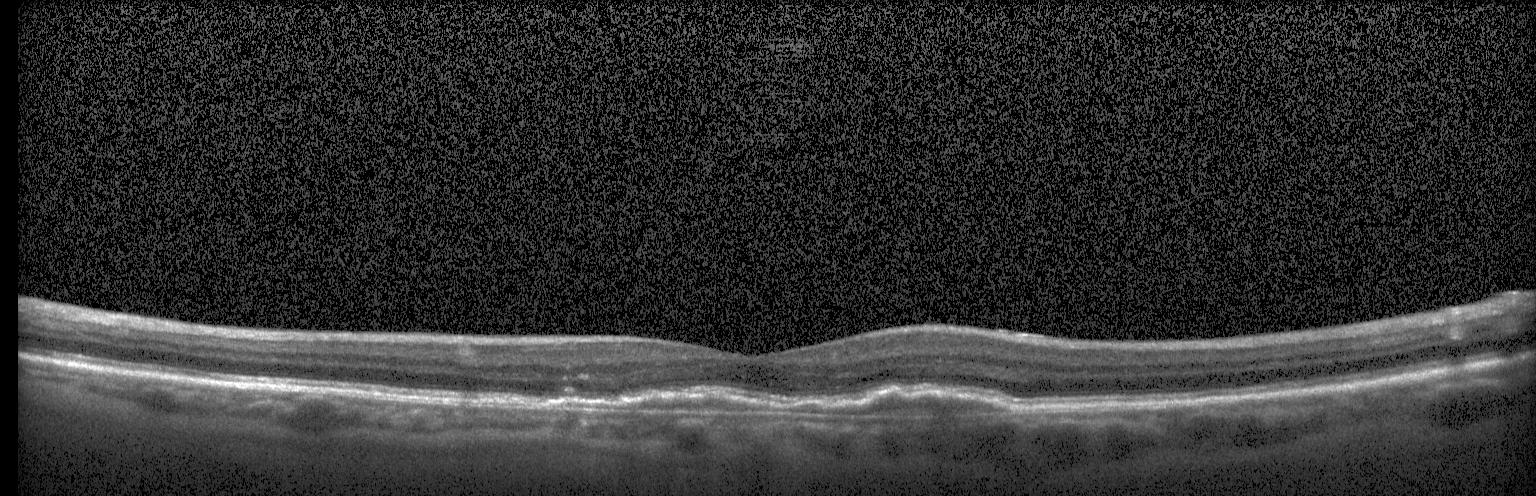
Instrument: Heidelberg Spectralis, optical coherence tomography scan, macular scan, spectral-domain optical coherence tomography.
This B-scan demonstrates CNV.